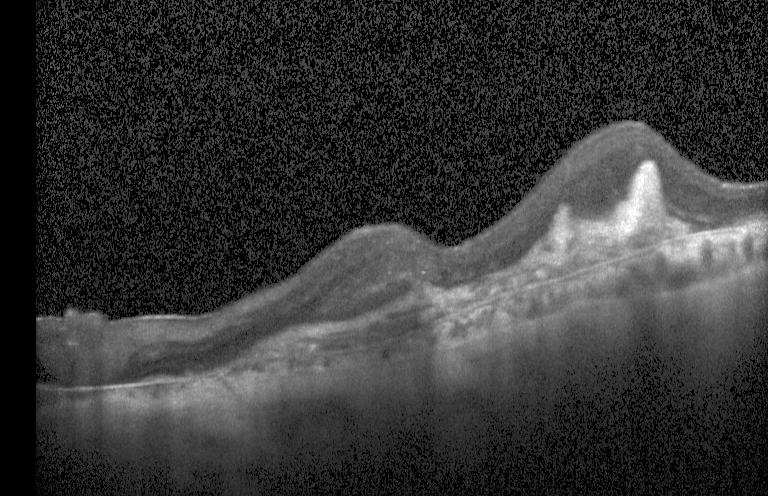 Optical coherence tomography scan. Instrument: Heidelberg Spectralis.
OCT finding: choroidal neovascularization (CNV).